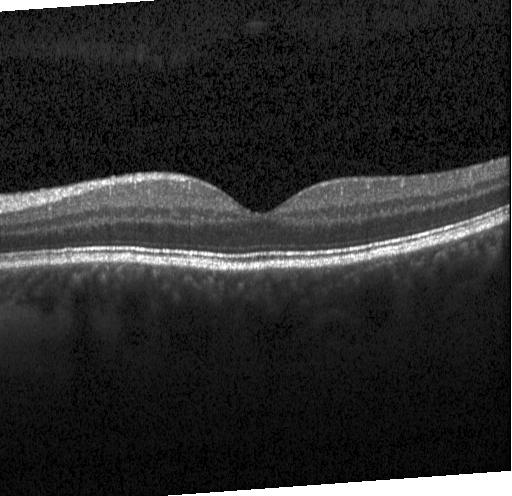

OCT line scan. Impression: no choroidal neovascularization, diabetic macular edema, or drusen.